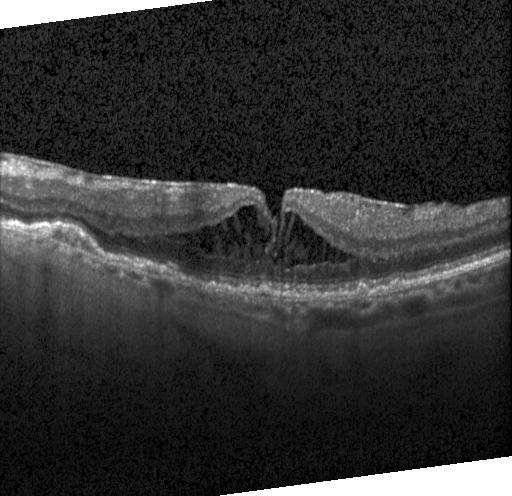
SD-OCT. Heidelberg Spectralis. OCT line scan. OCT finding: diabetic macular edema (DME).